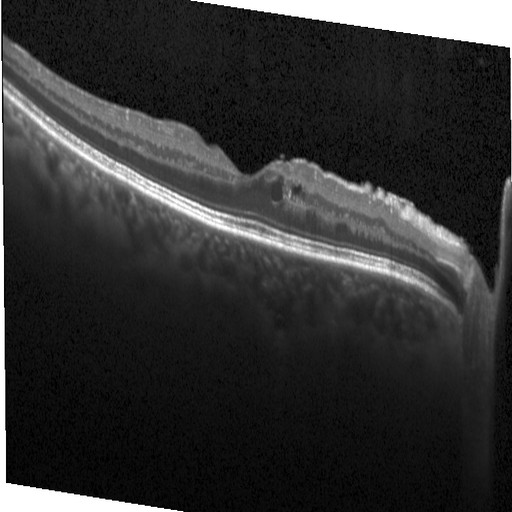 Spectral-domain OCT B-scan: diabetic macular edema.